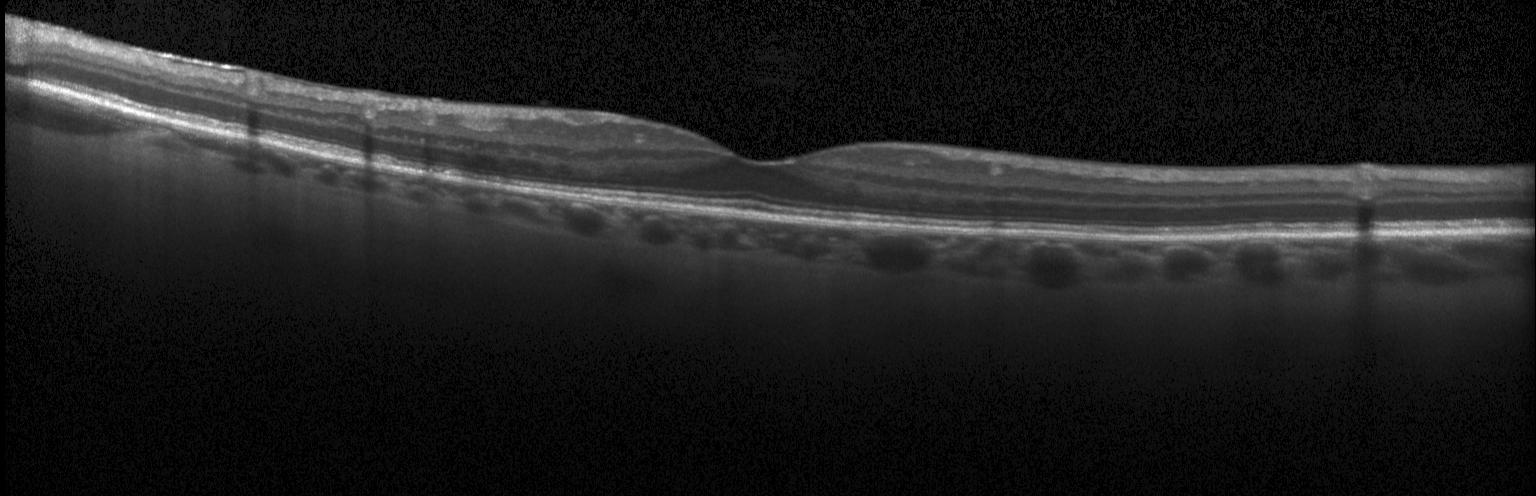
Optical coherence tomography B-scan; fovea-centered; Heidelberg Spectralis OCT system.
Dx: no choroidal neovascularization, diabetic macular edema, or drusen.